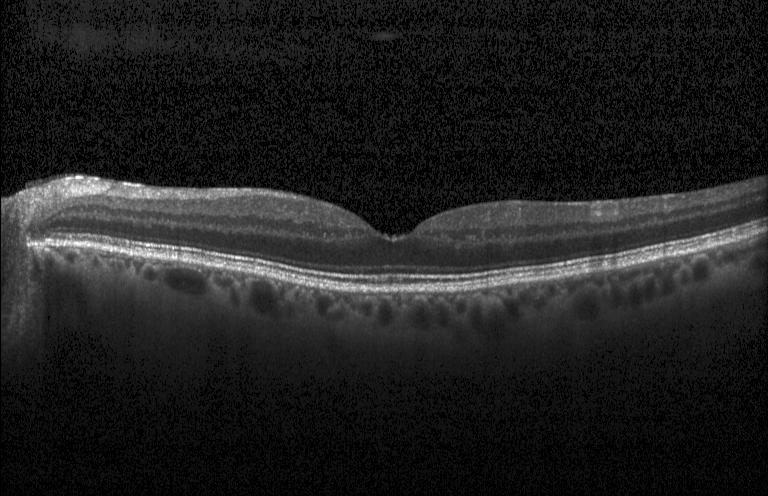

Retinal OCT B-scan.
Diagnosis: no choroidal neovascularization, diabetic macular edema, or drusen.